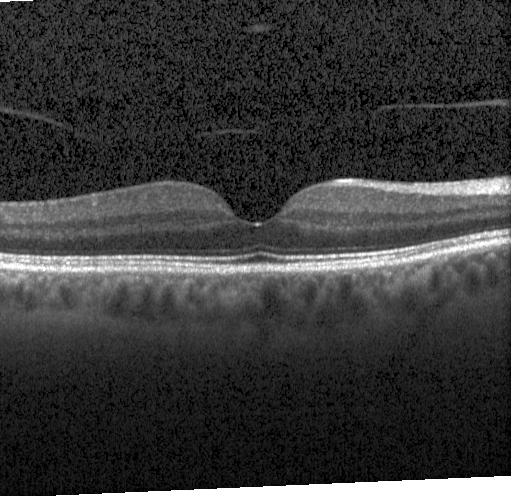 Acquired on a Heidelberg Spectralis; retinal OCT B-scan — Diagnosis: no CNV, DME, or drusen.